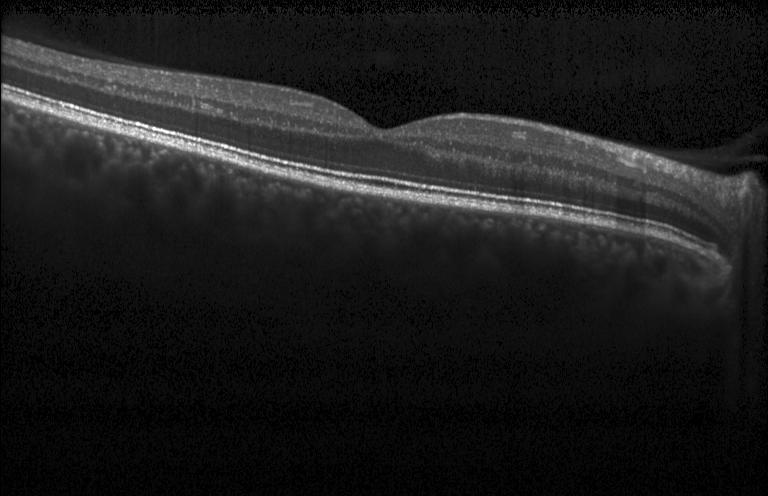

Heidelberg Spectralis, spectral-domain OCT, retinal OCT cross-section.
No evidence of choroidal neovascularization, diabetic macular edema, or drusen.